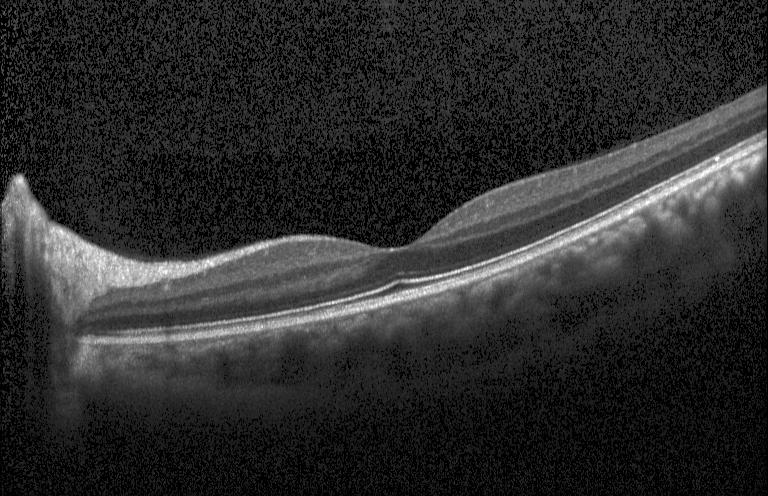

Optical coherence tomography scan; acquired on a Heidelberg Spectralis; centered on the fovea
Macular OCT: neither choroidal neovascularization, diabetic macular edema, nor drusen.